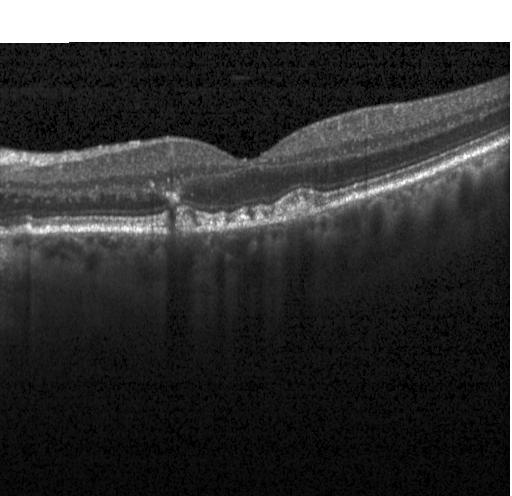 Finding: multiple drusen.